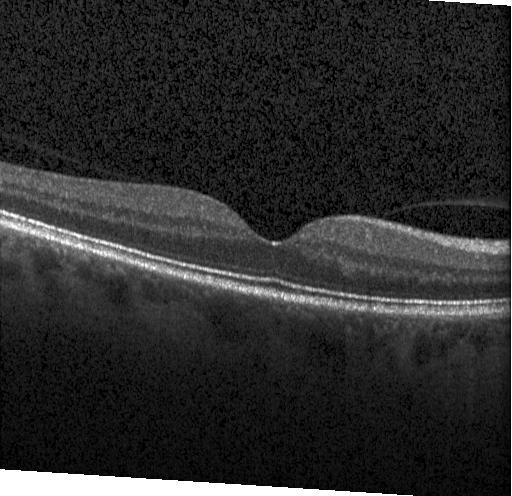 SD-OCT; retinal OCT B-scan — Dx: no evidence of choroidal neovascularization, diabetic macular edema, or drusen.